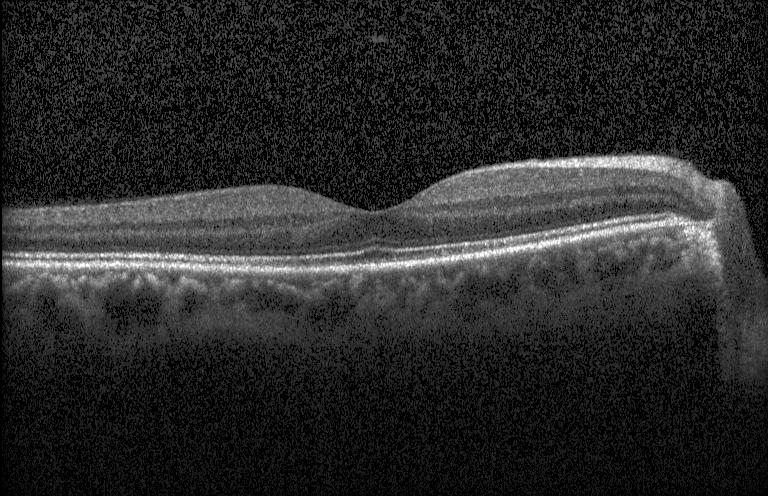
Impression: no evidence of choroidal neovascularization, diabetic macular edema, or drusen.